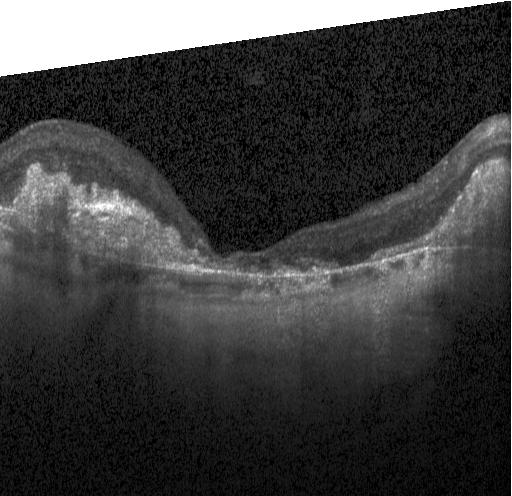 Retinal OCT cross-section. Horizontal scan through the fovea. Instrument: Heidelberg Spectralis — This B-scan demonstrates a choroidal neovascular membrane.